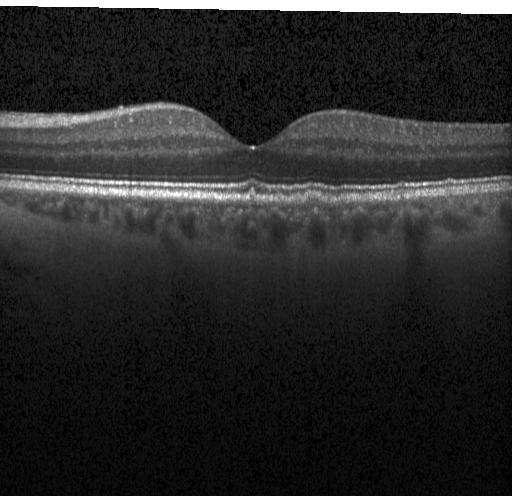

The scan shows multiple drusen.